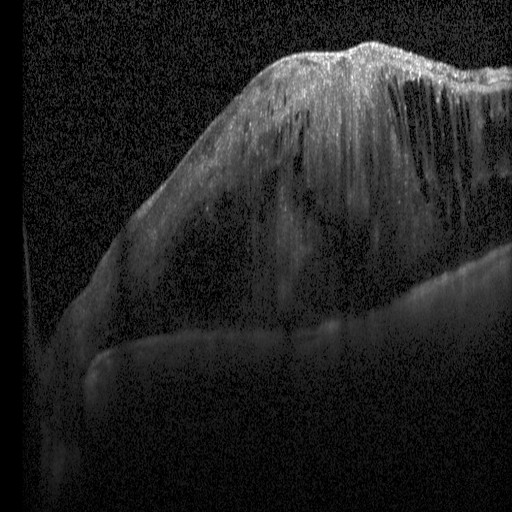 Spectral-domain OCT; OCT line scan. OCT finding: diabetic macular edema (DME).